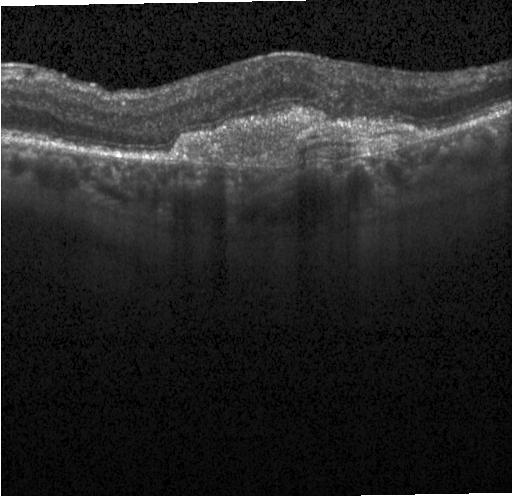
Heidelberg Spectralis · OCT line scan. Diagnosis: choroidal neovascularization.